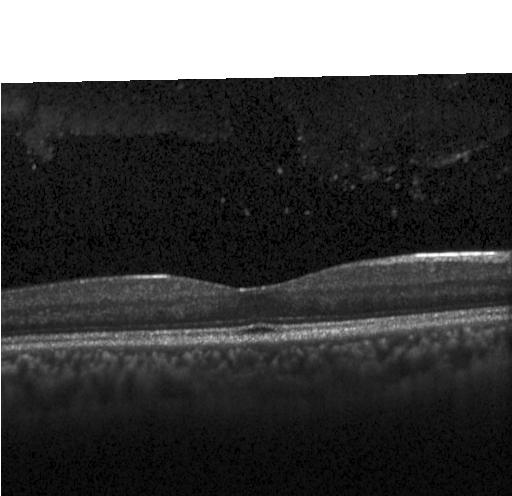 Macular OCT: no CNV, no DME, and no drusen.